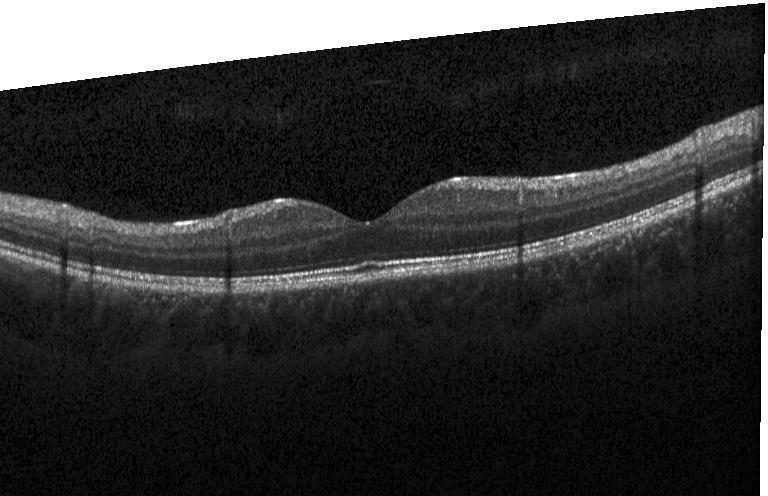
Retinal OCT cross-section — Macular OCT: neither choroidal neovascularization, diabetic macular edema, nor drusen.